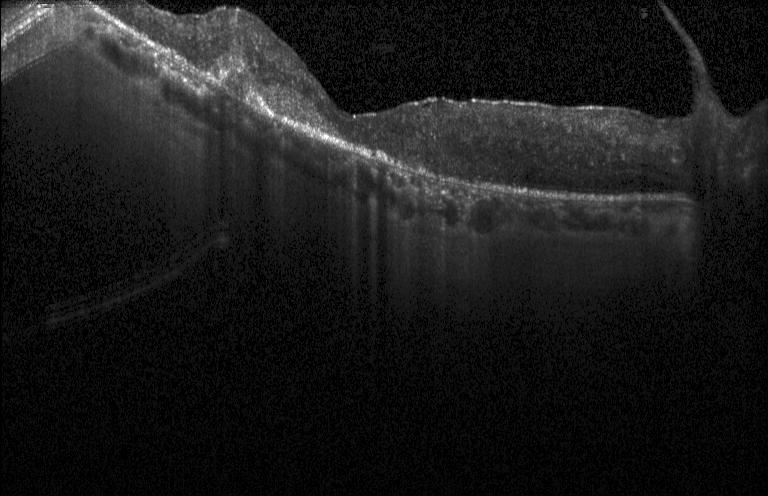 Spectral-domain OCT B-scan: CNV.